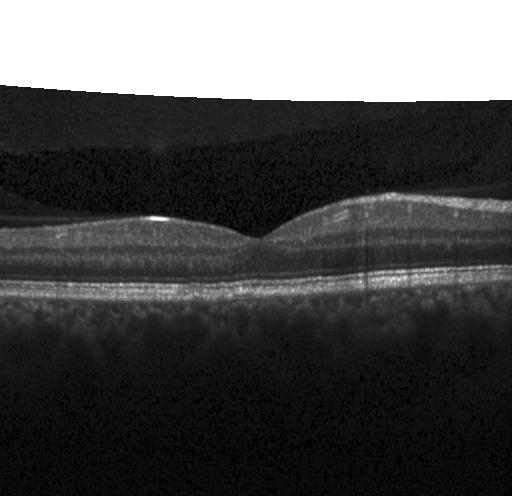 OCT B-scan. Centered on the fovea. Finding: neither choroidal neovascularization, diabetic macular edema, nor drusen.